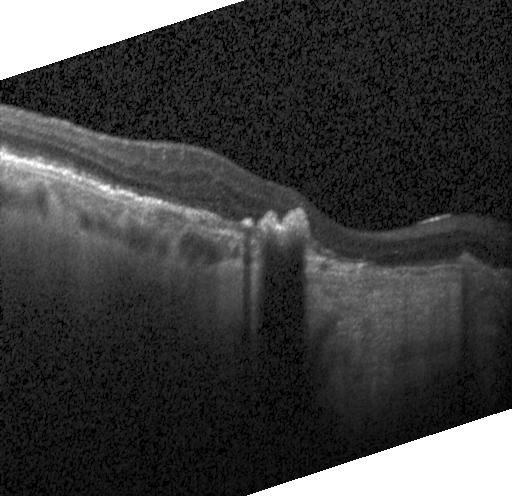

OCT scan showing choroidal neovascularization.